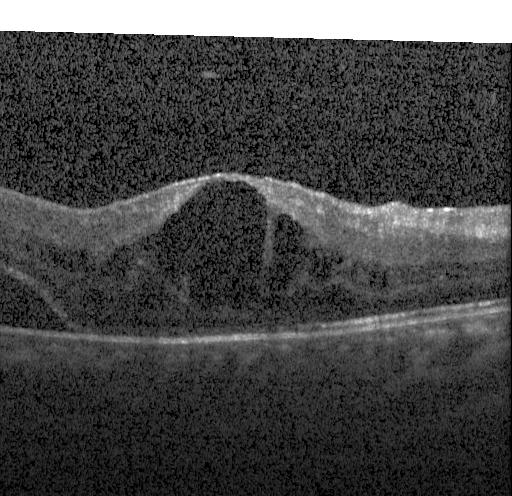
Optical coherence tomography B-scan · acquired on a Heidelberg Spectralis · SD-OCT · macular scan — Diabetic macular edema (DME).